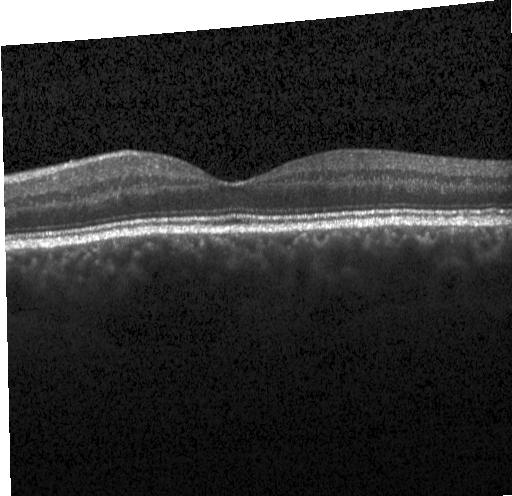 This B-scan demonstrates neither CNV, DME, nor drusen.